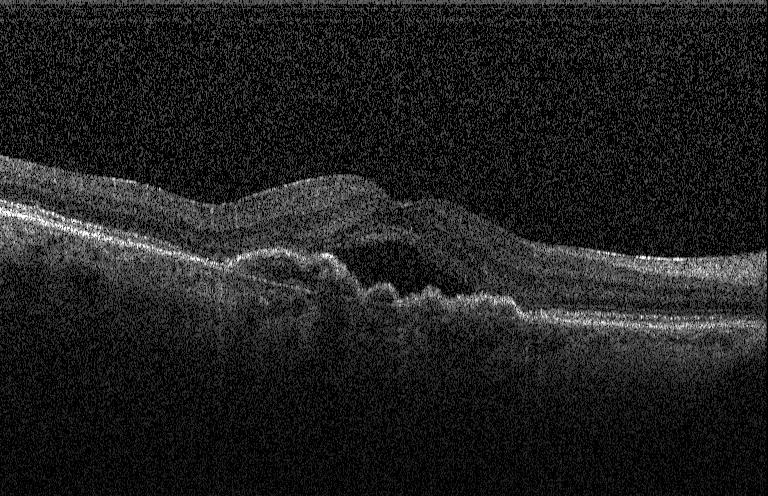 Spectral-domain optical coherence tomography. Optical coherence tomography scan. Heidelberg Spectralis OCT system — OCT finding: CNV.